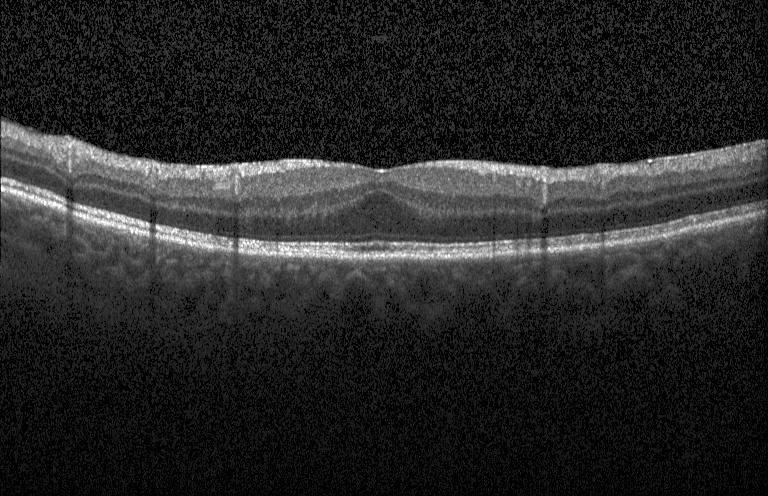
Impression: no CNV, DME, or drusen.